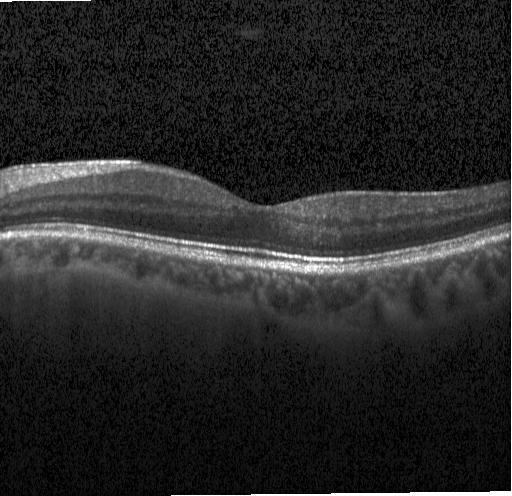
OCT B-scan showing no choroidal neovascularization, no diabetic macular edema, and no drusen.